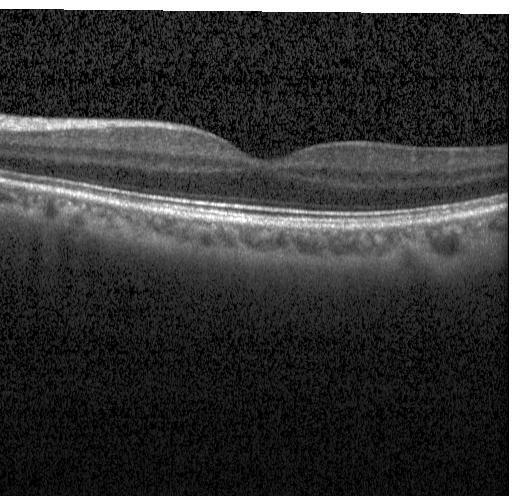

Diagnosis: neither choroidal neovascularization, diabetic macular edema, nor drusen.